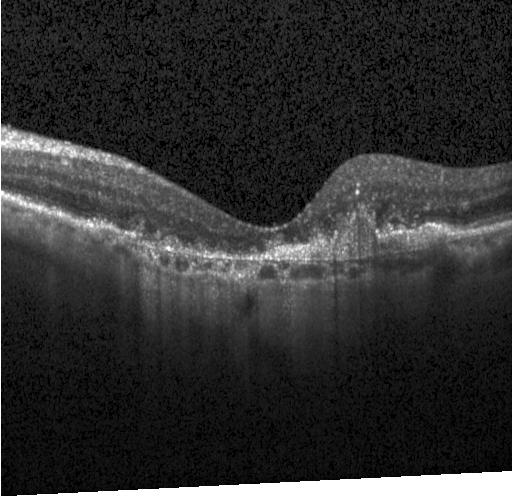
Retinal OCT cross-section, acquired on a Heidelberg Spectralis
Dx: a choroidal neovascular membrane.